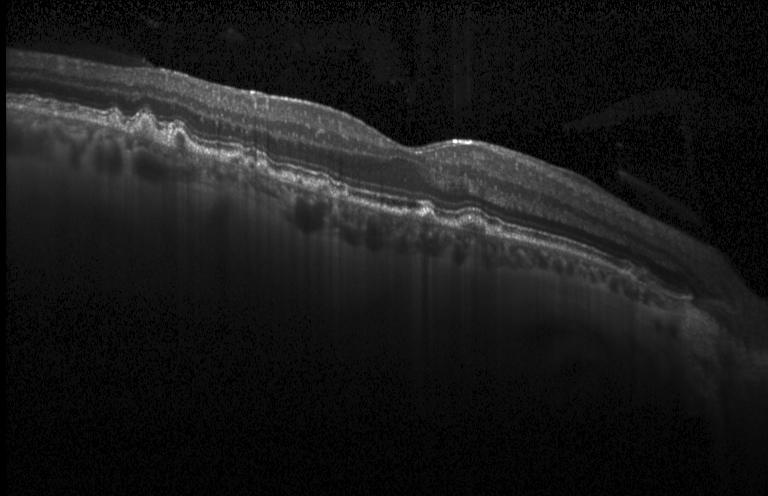
Optical coherence tomography scan. Spectral-domain optical coherence tomography. Heidelberg Spectralis. Impression: drusen.